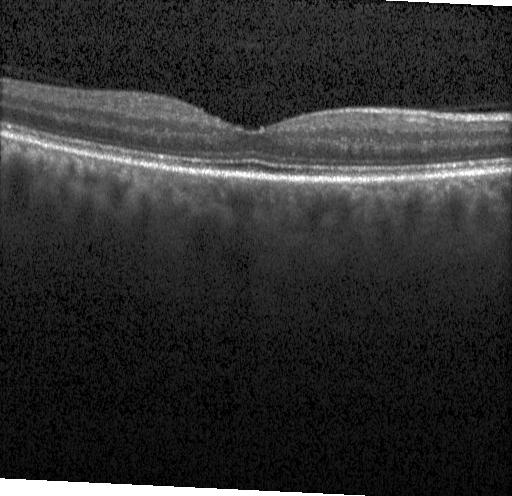
Assessment: no evidence of choroidal neovascularization, diabetic macular edema, or drusen.